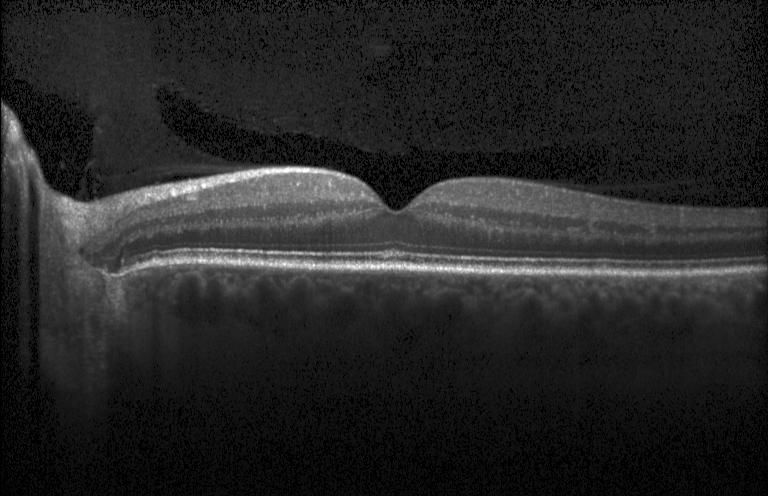 Retinal OCT cross-section — OCT finding: neither CNV, DME, nor drusen.